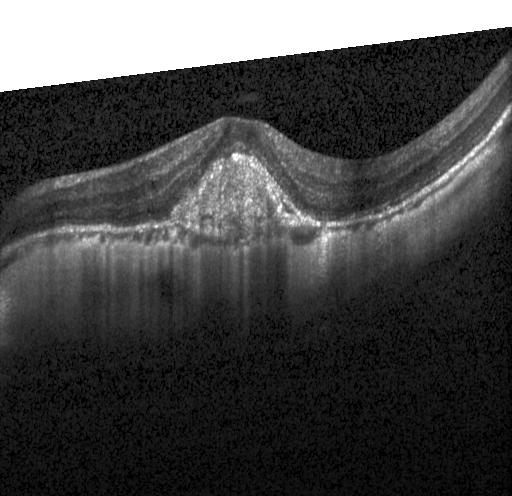
Choroidal neovascularization.